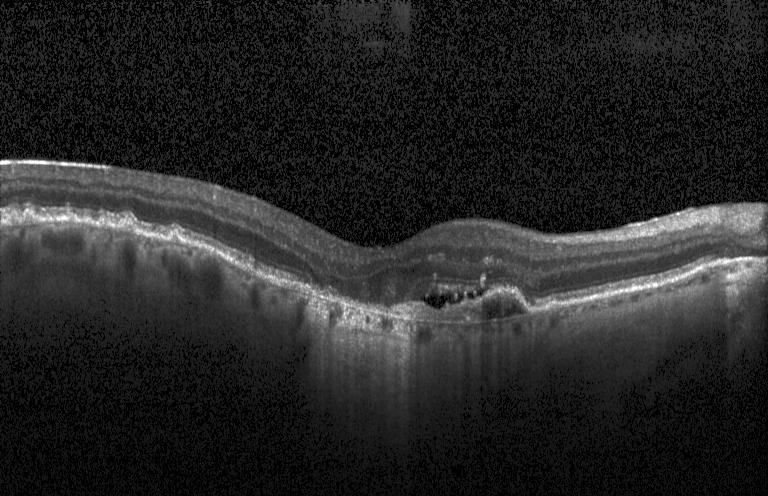
Finding: a choroidal neovascular membrane.